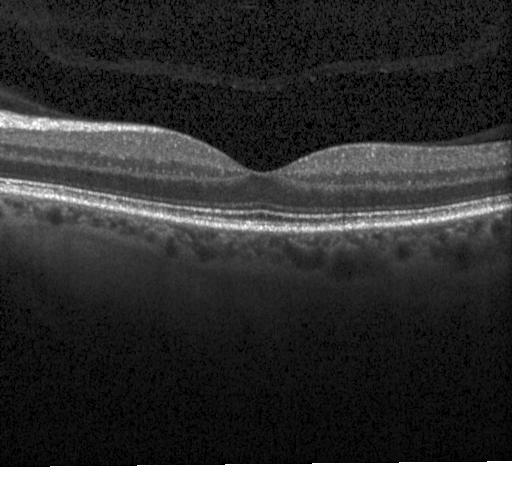 Horizontal scan through the fovea. Spectral-domain OCT. OCT line scan. Acquired on a Heidelberg Spectralis.
Finding: no evidence of choroidal neovascularization, diabetic macular edema, or drusen.